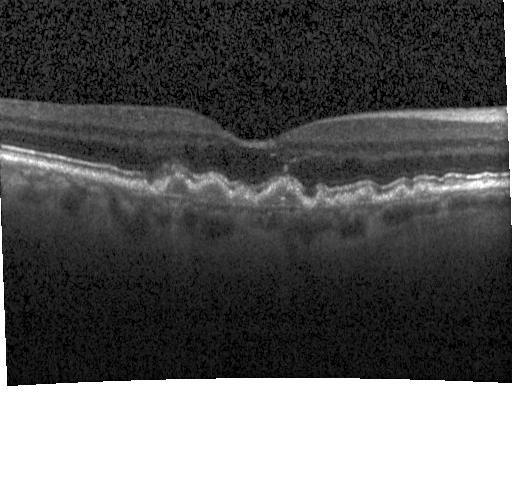
Optical coherence tomography B-scan · instrument: Heidelberg Spectralis · spectral-domain OCT · fovea-centered.
Diagnosis: drusen.